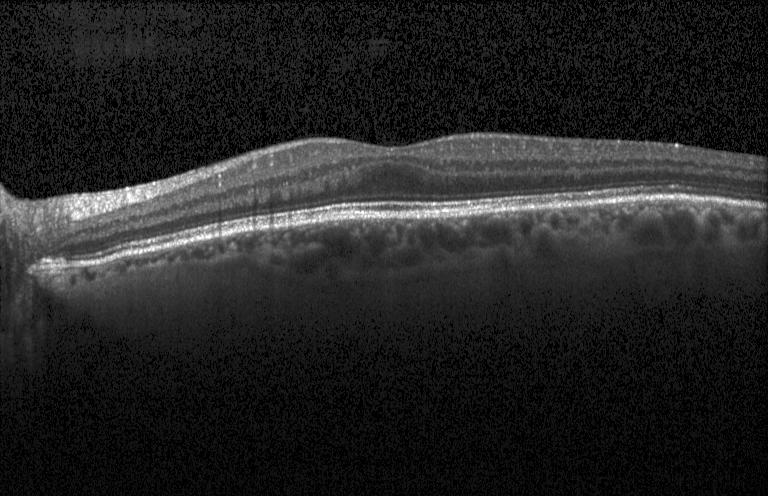

Optical coherence tomography scan; acquired on a Heidelberg Spectralis; through the macula. Impression: no CNV, DME, or drusen.